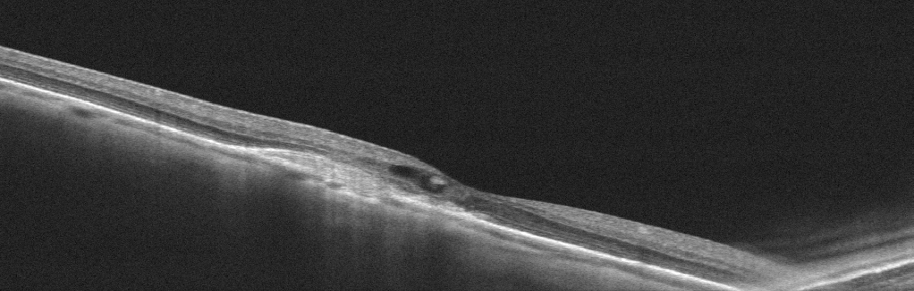
Optovue Avanti RTVue XR; optical coherence tomography B-scan.
Diagnosis: AMD.